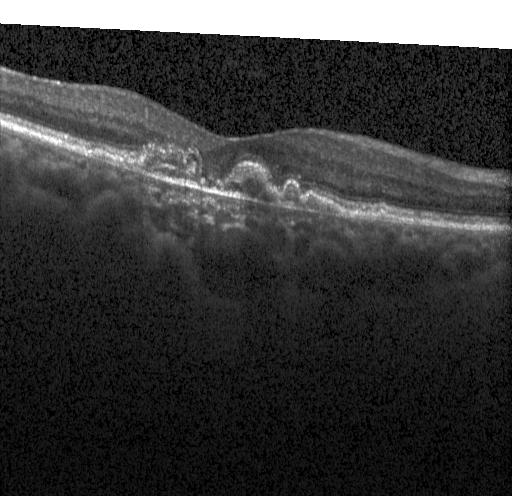

Finding: a choroidal neovascular membrane.